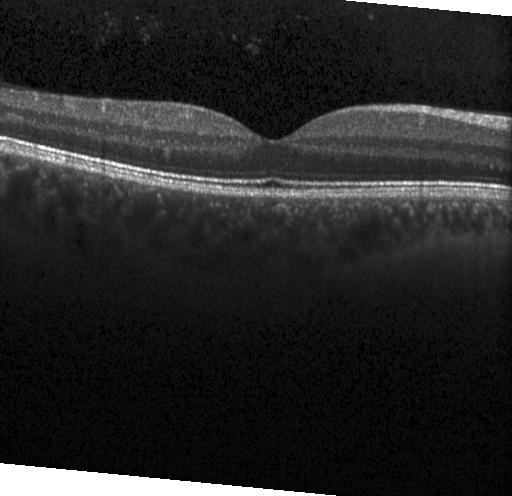
Instrument: Heidelberg Spectralis · horizontal scan through the fovea · OCT B-scan · SD-OCT.
No choroidal neovascularization, no diabetic macular edema, and no drusen.